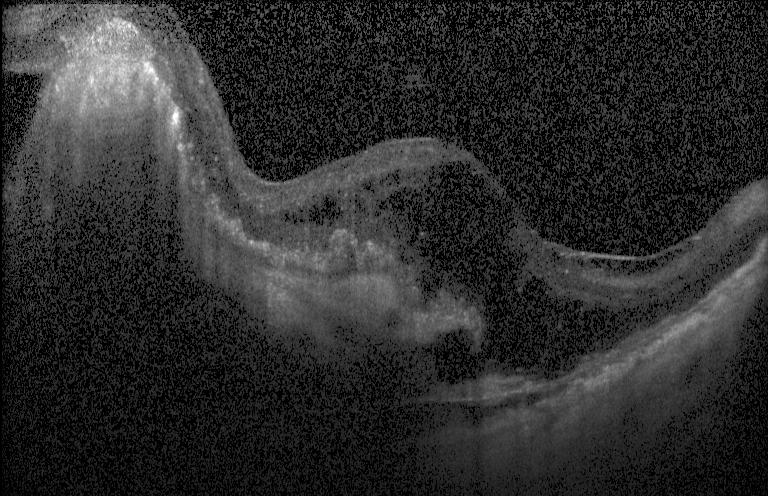 Macular OCT demonstrating a choroidal neovascular membrane.